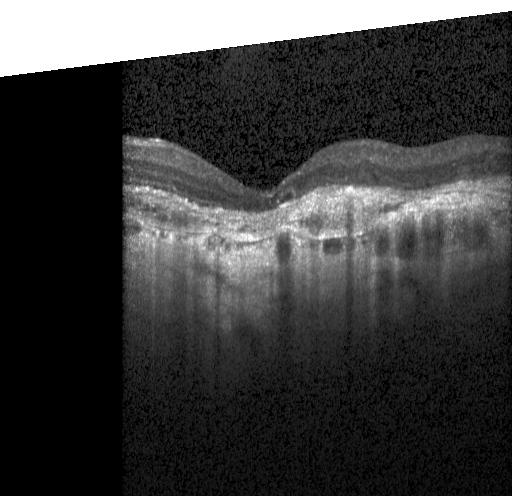 Acquired on a Heidelberg Spectralis. OCT line scan. This B-scan demonstrates choroidal neovascularization (CNV).